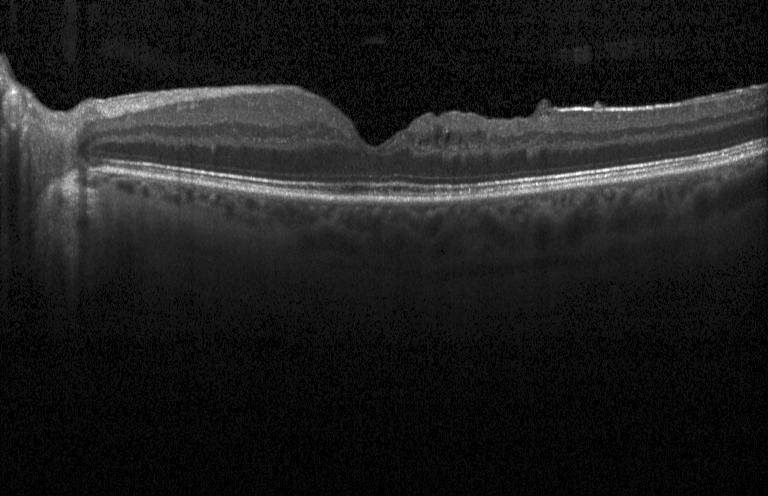

Heidelberg Spectralis OCT system · retinal OCT cross-section · horizontal scan through the fovea. OCT finding: diabetic macular edema (DME).